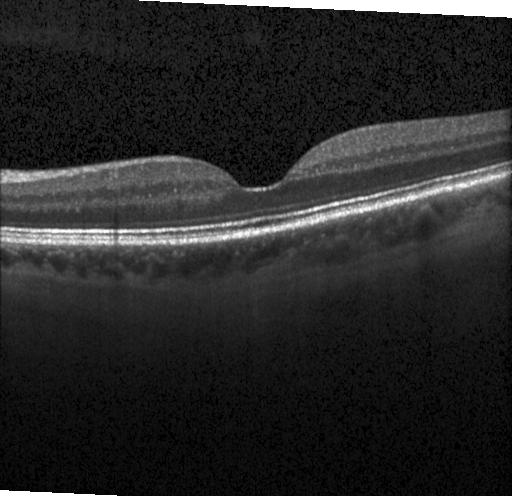
OCT finding: no evidence of choroidal neovascularization, diabetic macular edema, or drusen.